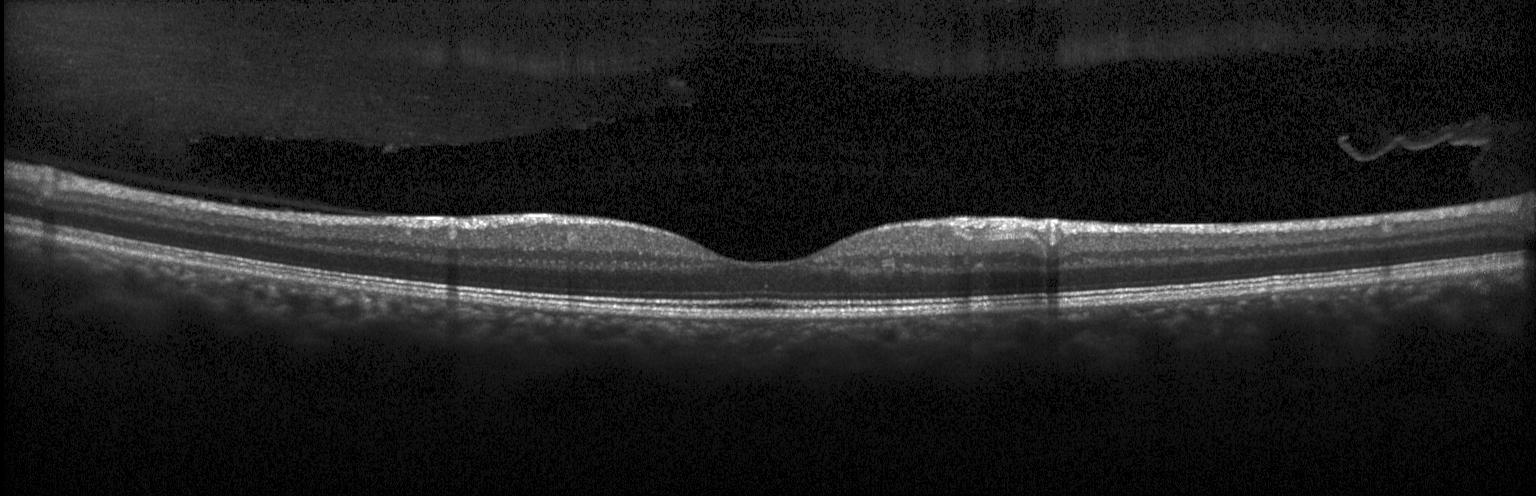
Finding: no choroidal neovascularization, diabetic macular edema, or drusen.